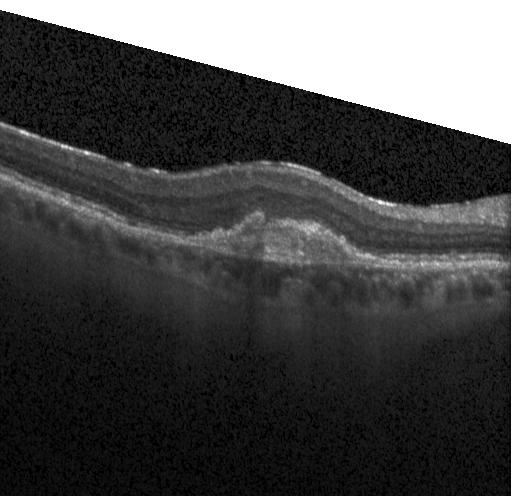
Dx: CNV.